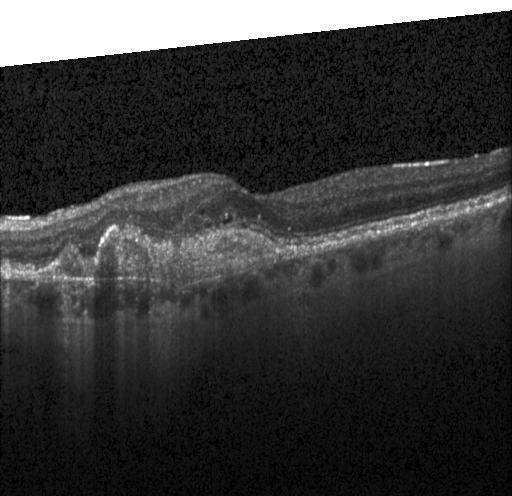 Retinal OCT B-scan; fovea-centered; SD-OCT.
Assessment: CNV.